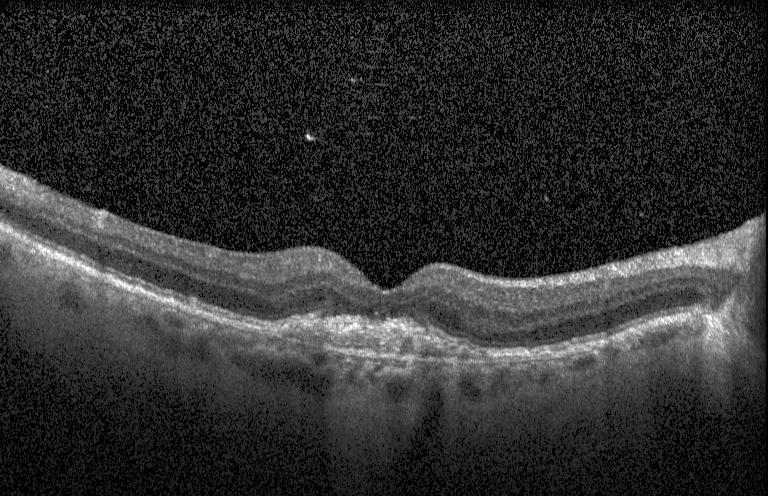 SD-OCT; retinal OCT B-scan; fovea-centered; instrument: Heidelberg Spectralis. This B-scan demonstrates a choroidal neovascular membrane.